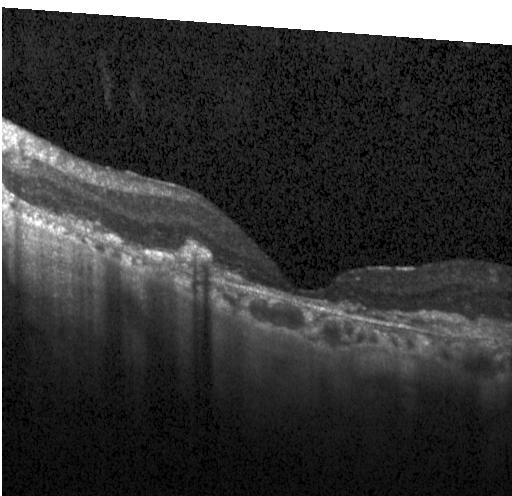 OCT scan showing choroidal neovascularization (CNV).